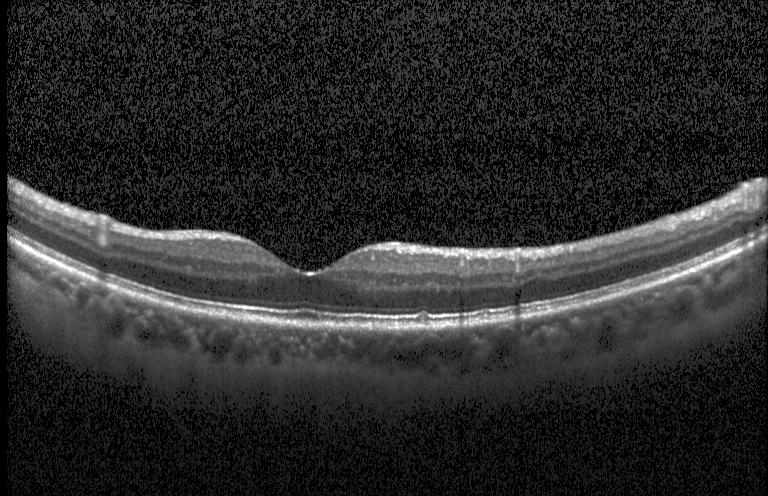
Optical coherence tomography scan. SD-OCT. Horizontal scan through the fovea. Instrument: Heidelberg Spectralis.
Impression: no evidence of choroidal neovascularization, diabetic macular edema, or drusen.